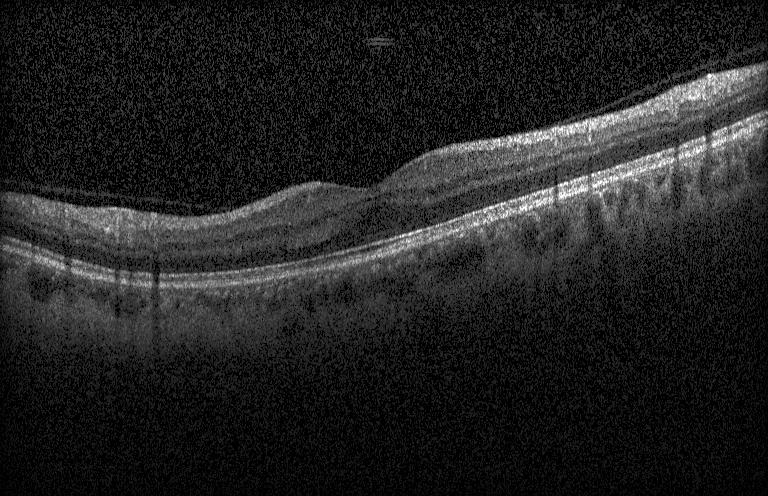 Spectral-domain OCT B-scan: no choroidal neovascularization, diabetic macular edema, or drusen.